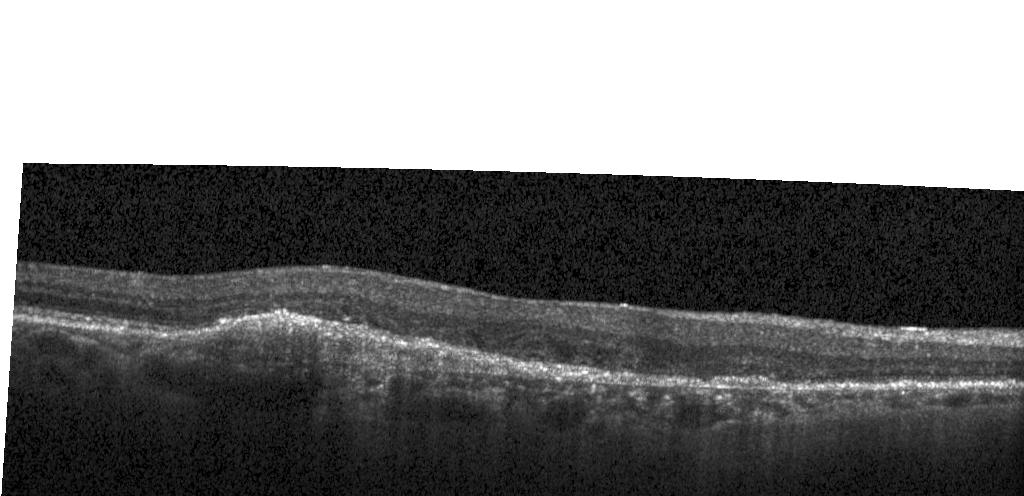

Macular OCT demonstrating choroidal neovascularization.